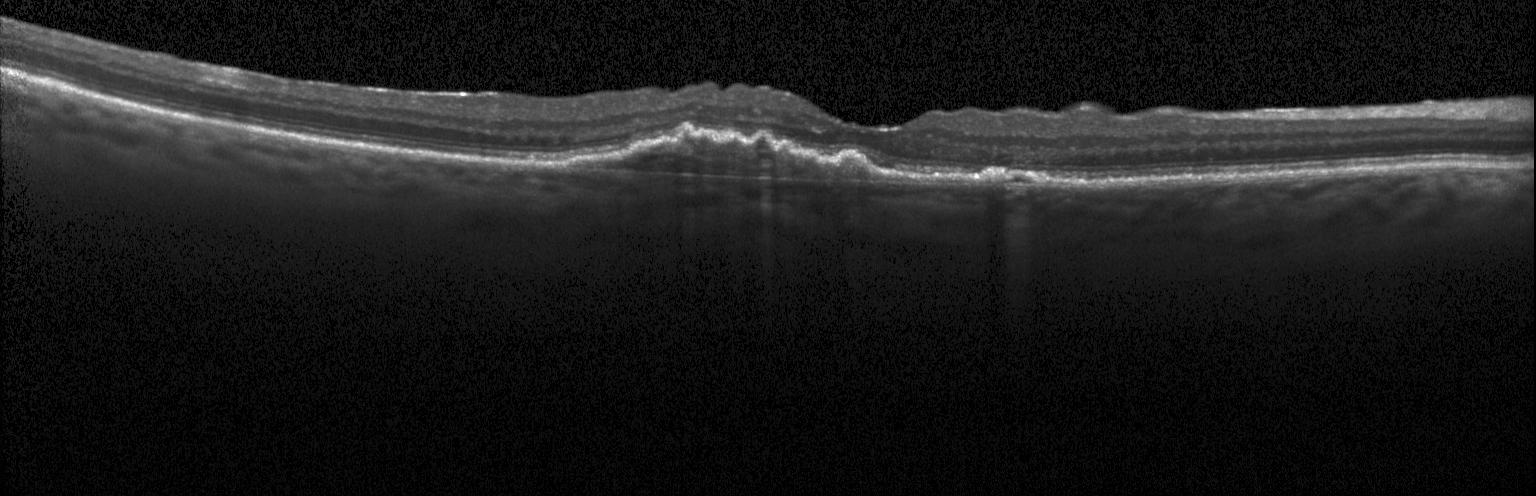

Heidelberg Spectralis, OCT line scan
This B-scan demonstrates choroidal neovascularization (CNV).